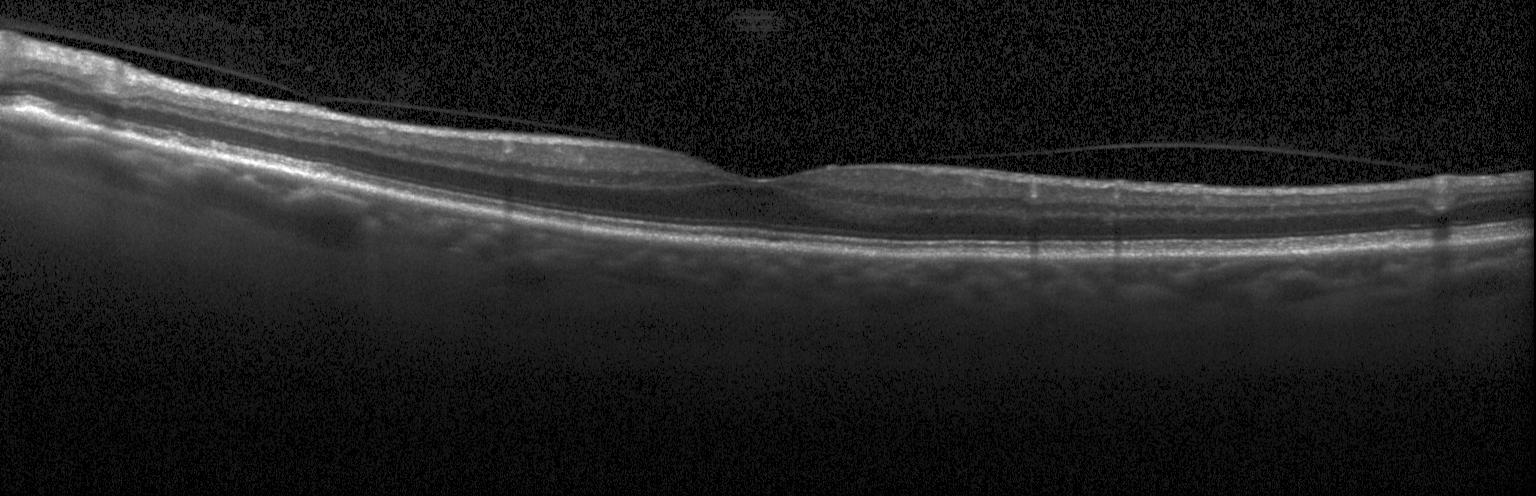 OCT line scan · SD-OCT · centered on the fovea · Heidelberg Spectralis
Diagnosis: neither CNV, DME, nor drusen.